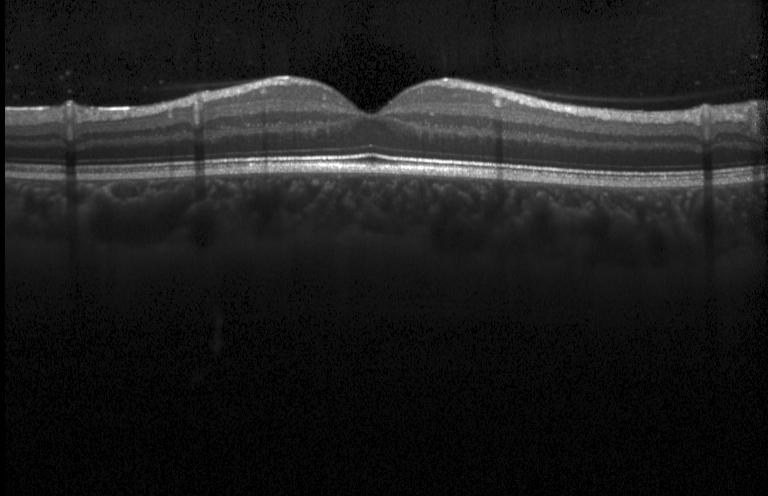

Optical coherence tomography B-scan · Heidelberg Spectralis OCT system — Diagnosis: no choroidal neovascularization, diabetic macular edema, or drusen.